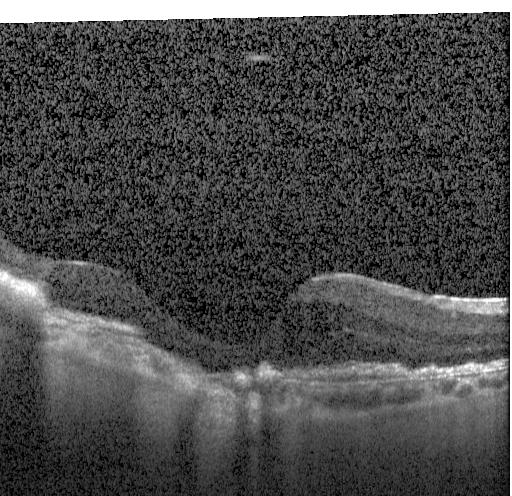 Diagnosis: choroidal neovascularization.